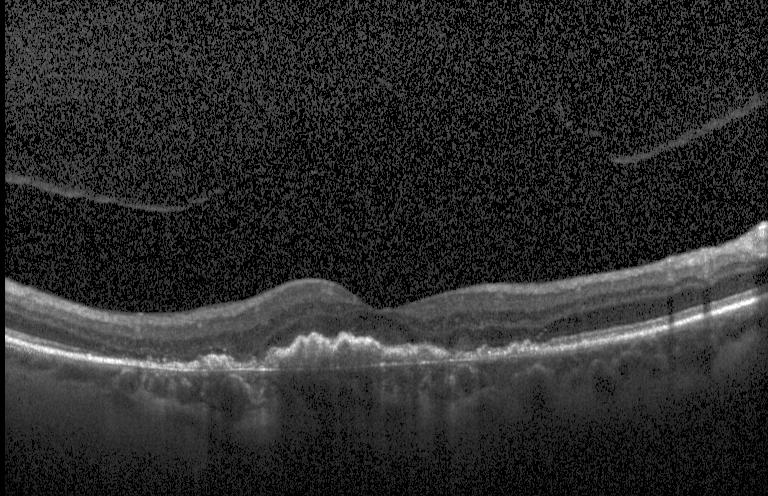
Spectral-domain OCT, macular scan, retinal OCT cross-section, Heidelberg Spectralis — Diagnosis: a choroidal neovascular membrane.